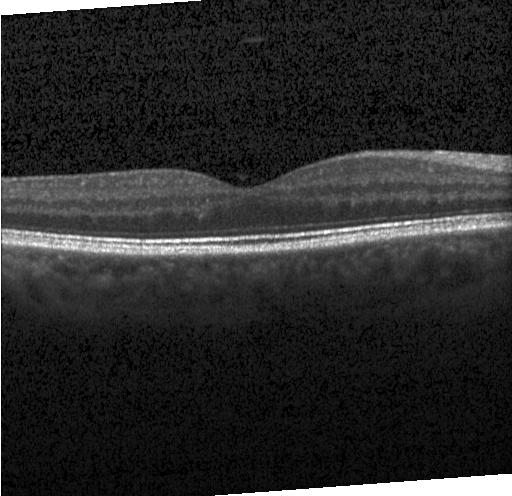 Retinal OCT cross-section; fovea-centered; SD-OCT; instrument: Heidelberg Spectralis — Impression: no choroidal neovascularization, no diabetic macular edema, and no drusen.